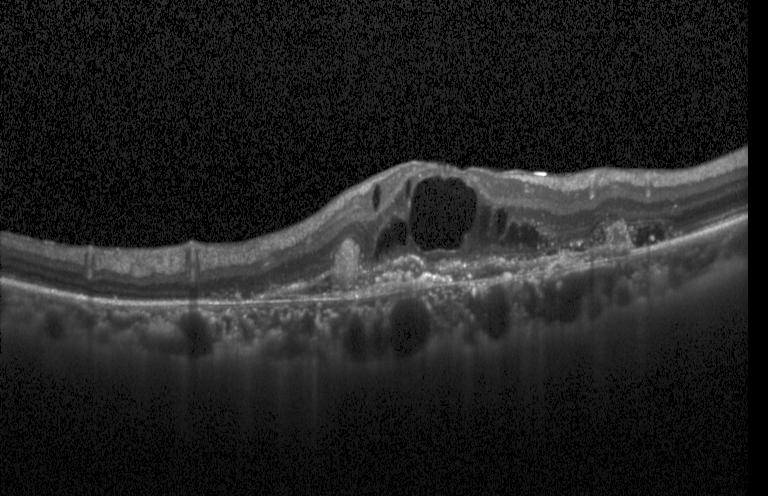 Diagnosis: choroidal neovascularization (CNV).